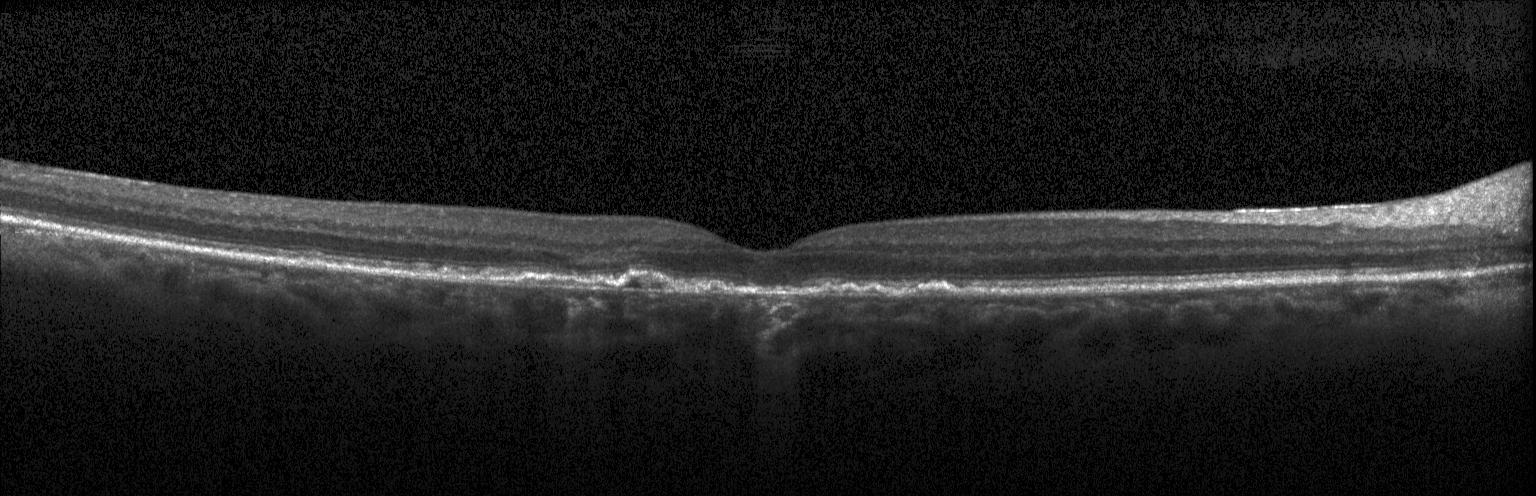 SD-OCT; optical coherence tomography scan; Heidelberg Spectralis OCT system.
Macular OCT: choroidal neovascularization.